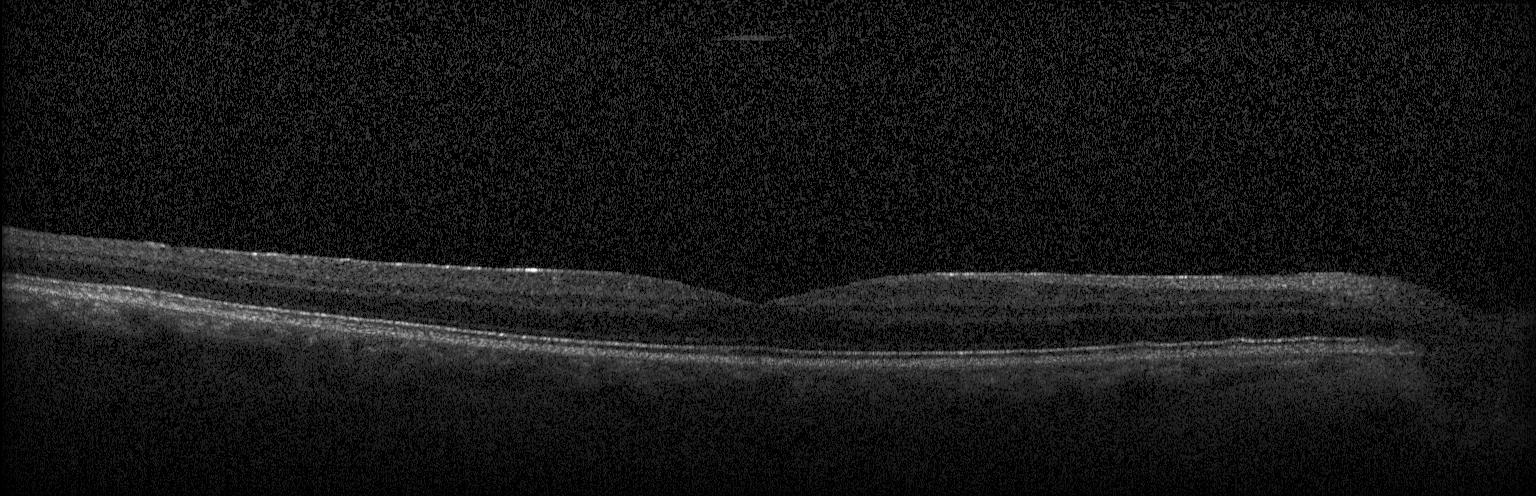
Optical coherence tomography B-scan; Heidelberg Spectralis; macular scan
Diagnosis: no evidence of CNV, DME, or drusen.